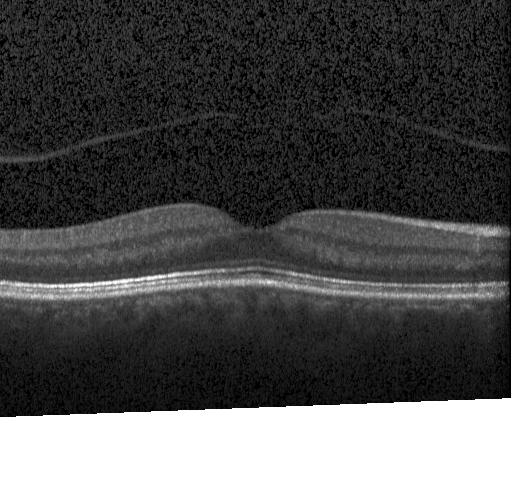
OCT B-scan
Finding: no CNV, no DME, and no drusen.